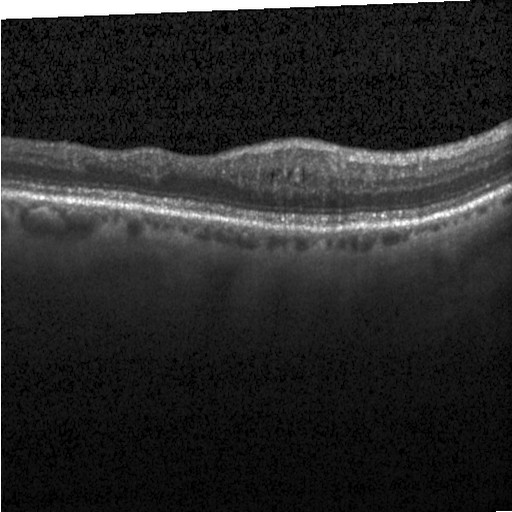 OCT line scan. Spectral-domain OCT
Impression: diabetic macular edema (DME).